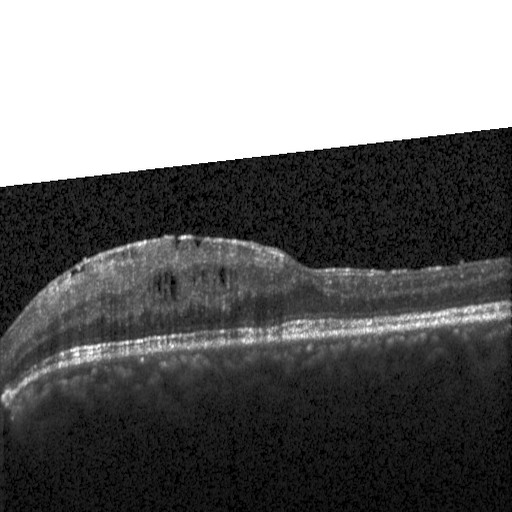 Macular OCT demonstrating DME.